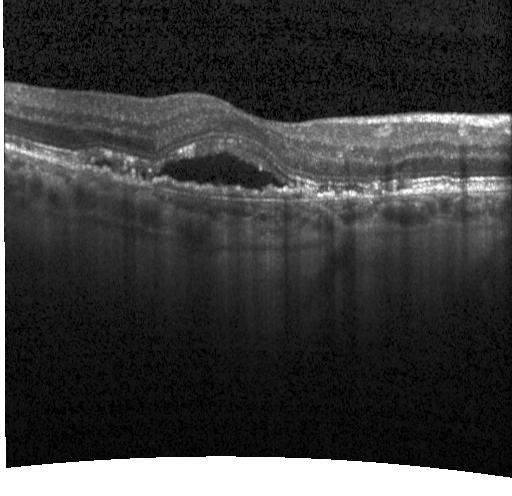
Diagnosis: CNV.